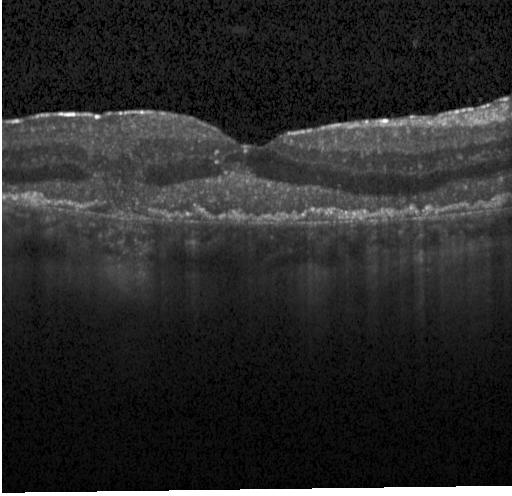

This B-scan demonstrates choroidal neovascularization.